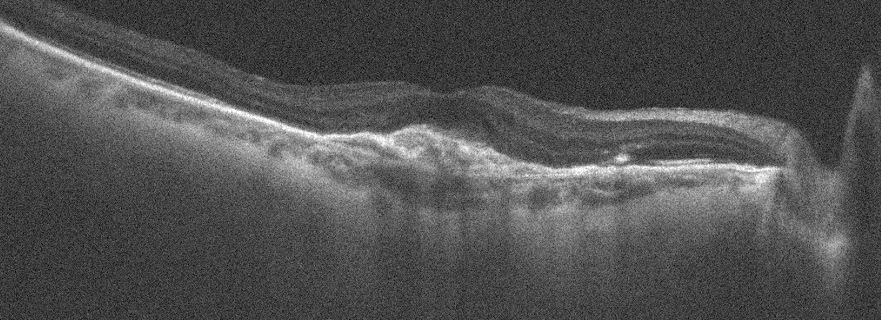
Spectral-domain OCT B-scan: age-related macular degeneration.